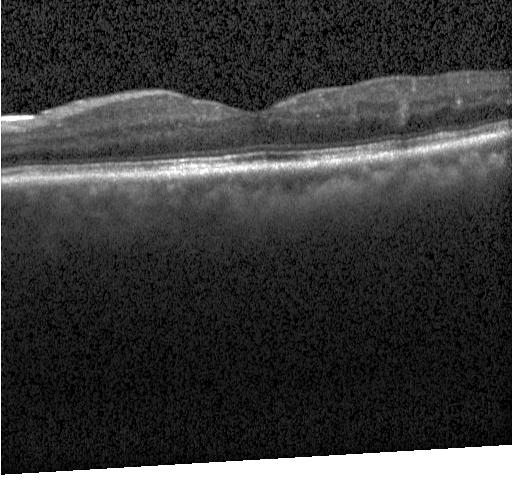
SD-OCT. Retinal OCT B-scan. Instrument: Heidelberg Spectralis — This B-scan demonstrates neither CNV, DME, nor drusen.